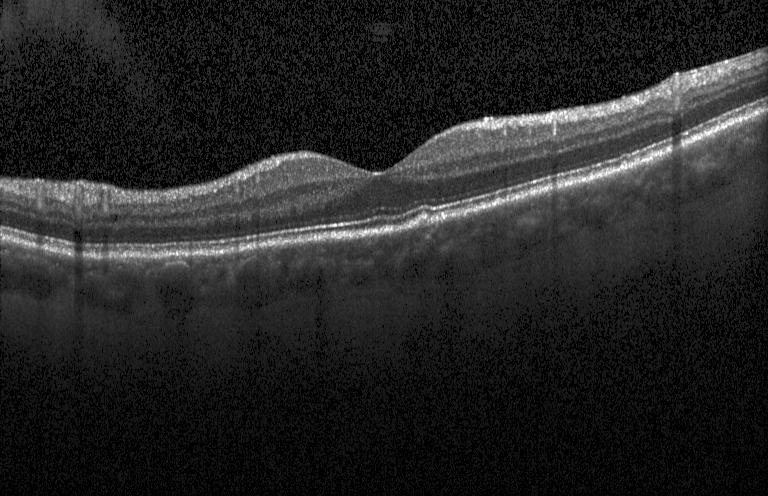 Retinal OCT cross-section showing multiple drusen.